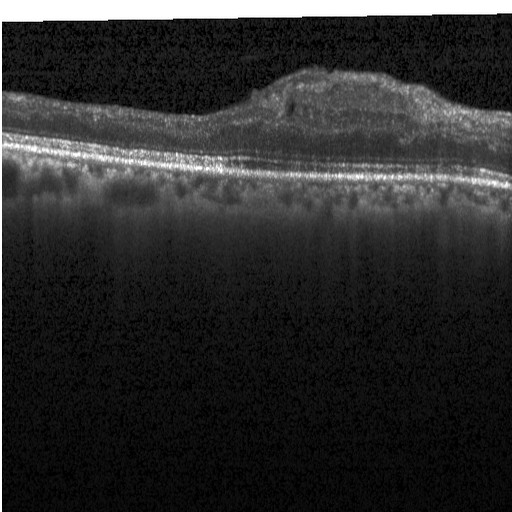
Diagnosis: DME.